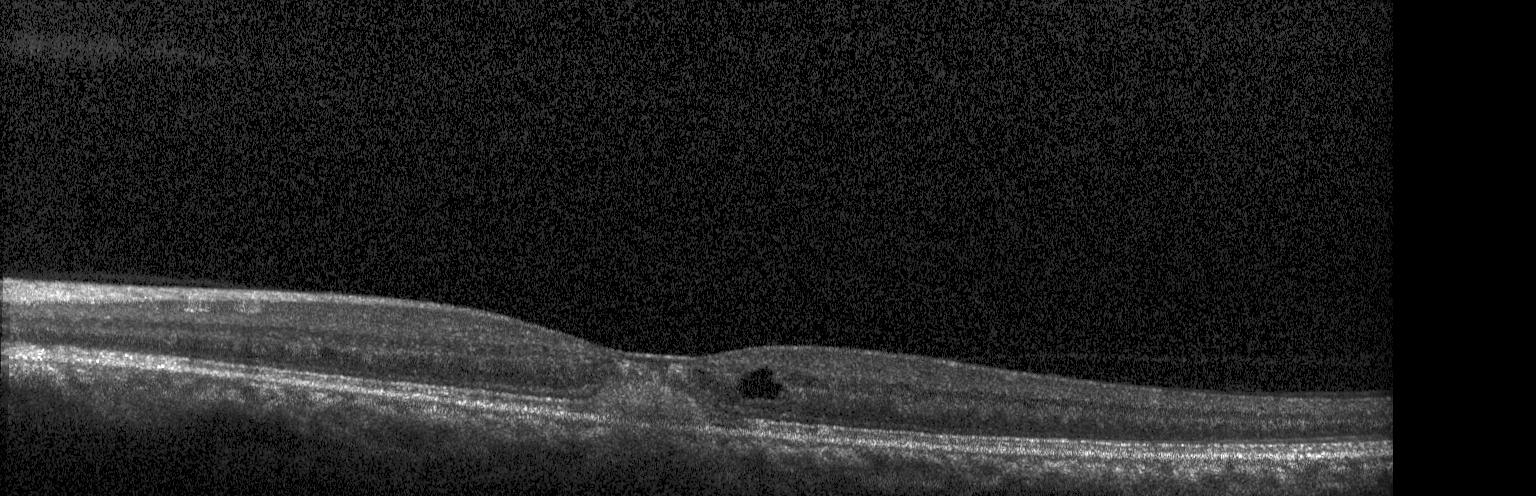 Through the macula · acquired on a Heidelberg Spectralis · SD-OCT · OCT line scan — Macular OCT: choroidal neovascularization.